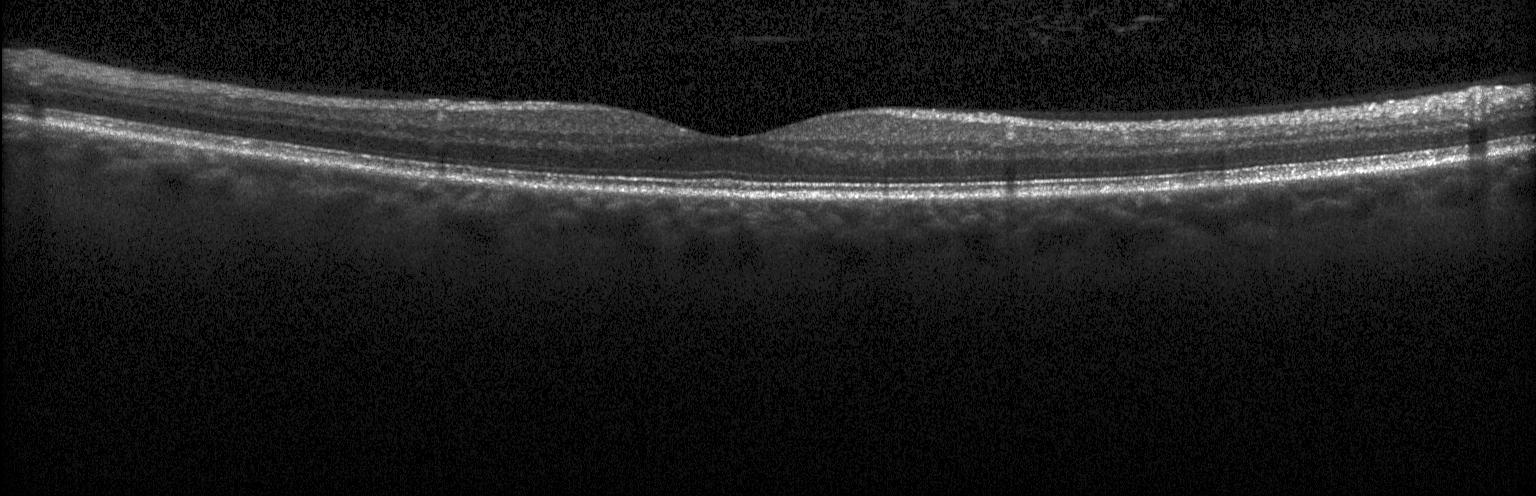
OCT B-scan · Heidelberg Spectralis · spectral-domain optical coherence tomography — Assessment: no choroidal neovascularization, no diabetic macular edema, and no drusen.